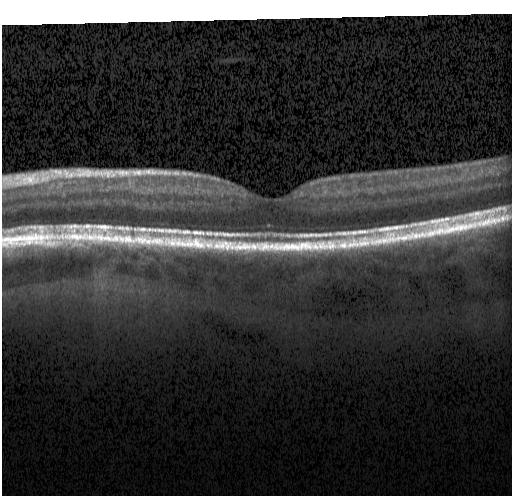
Fovea-centered · OCT B-scan — This B-scan demonstrates neither choroidal neovascularization, diabetic macular edema, nor drusen.